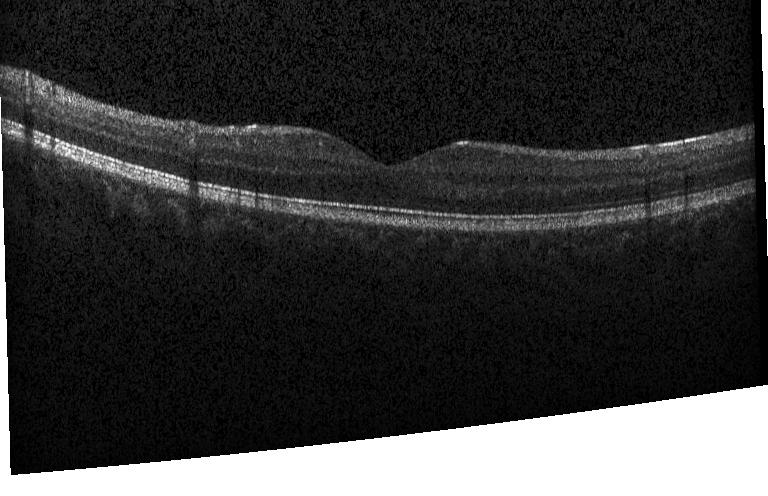
OCT B-scan showing no choroidal neovascularization, no diabetic macular edema, and no drusen.